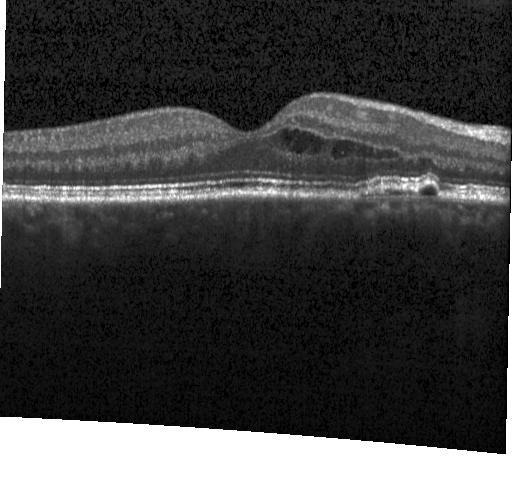

Through the macula; optical coherence tomography scan — Assessment: a choroidal neovascular membrane.